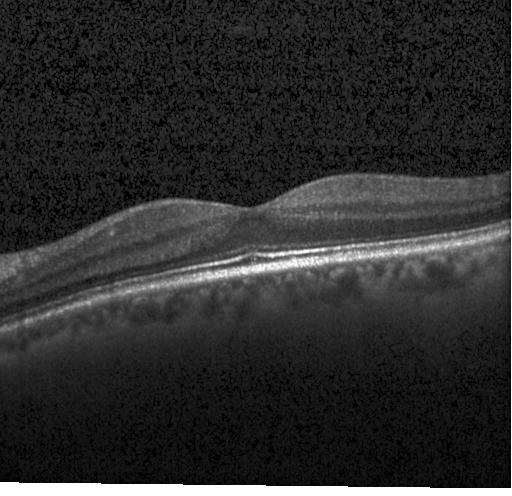

Diagnosis: no CNV, no DME, and no drusen.